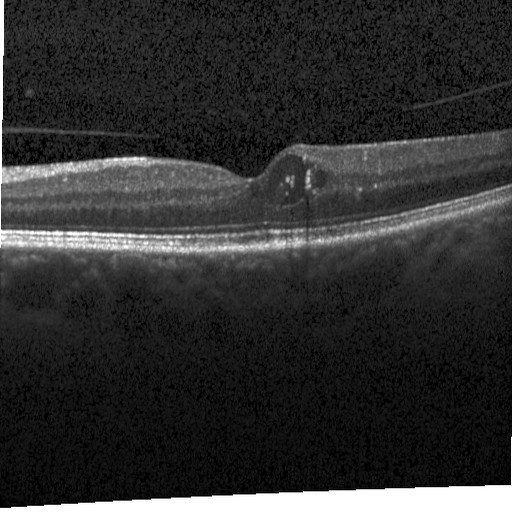 Retinal OCT B-scan · instrument: Heidelberg Spectralis — Finding: DME.